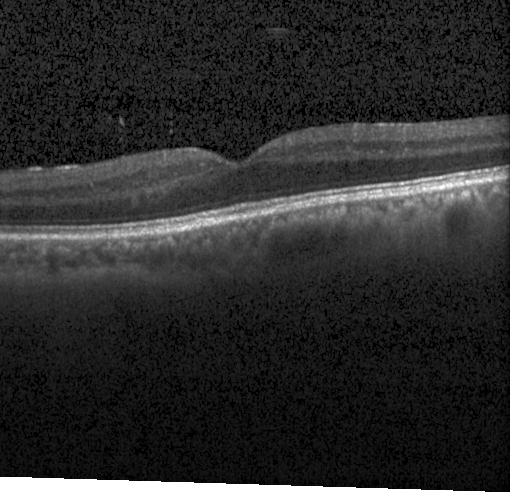

Retinal OCT B-scan, SD-OCT. Impression: no choroidal neovascularization, no diabetic macular edema, and no drusen.